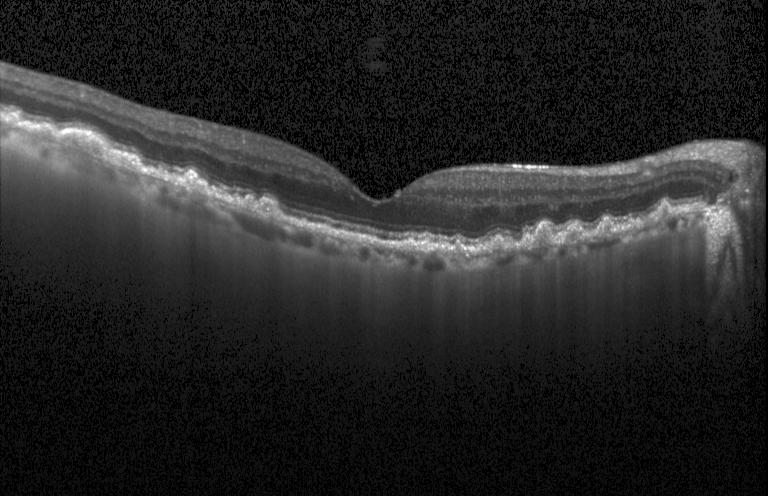
SD-OCT. Instrument: Heidelberg Spectralis. Retinal OCT cross-section. Horizontal scan through the fovea
This B-scan demonstrates drusen.